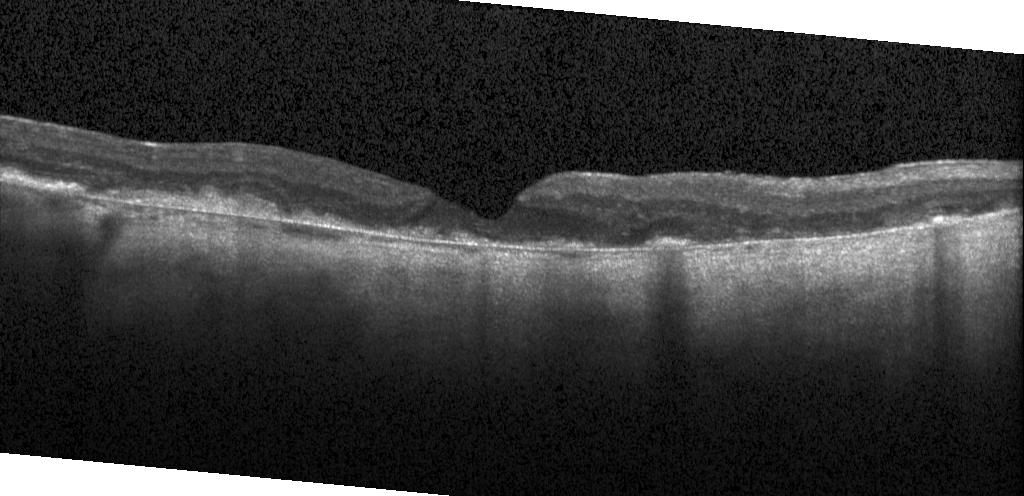 Spectral-domain OCT. Fovea-centered. OCT line scan. Choroidal neovascularization.